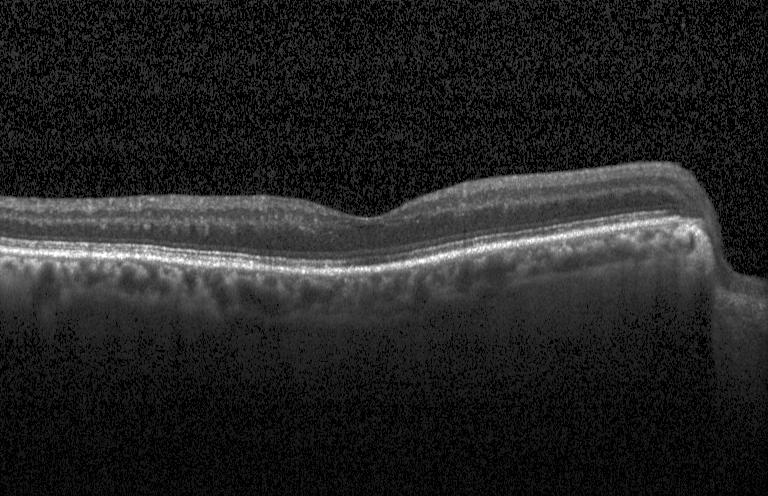 The scan shows no evidence of choroidal neovascularization, diabetic macular edema, or drusen.